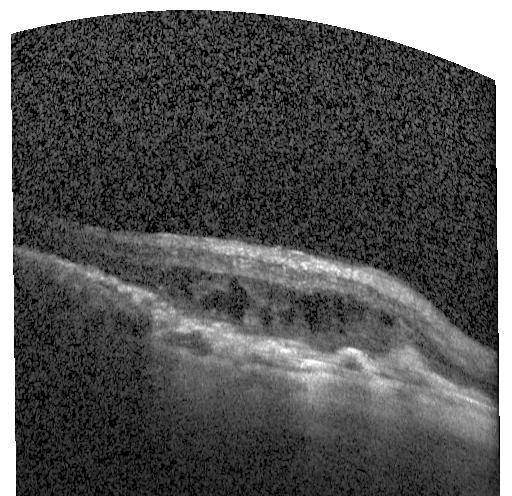 Optical coherence tomography scan
OCT finding: a choroidal neovascular membrane.